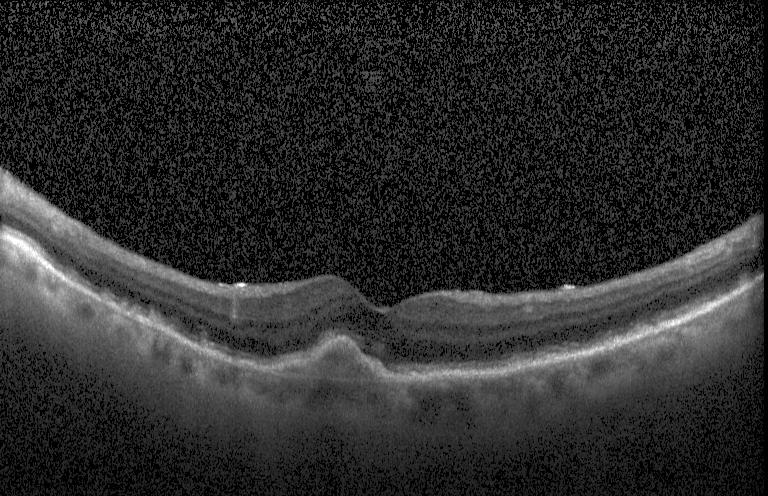

SD-OCT. Acquired on a Heidelberg Spectralis. Macular scan. OCT line scan. The scan shows a choroidal neovascular membrane.